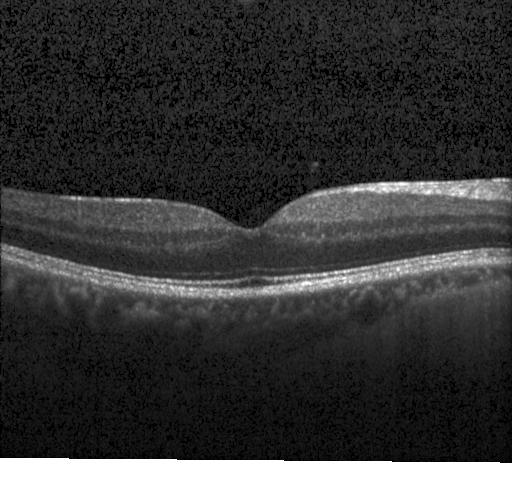 Finding: neither CNV, DME, nor drusen.